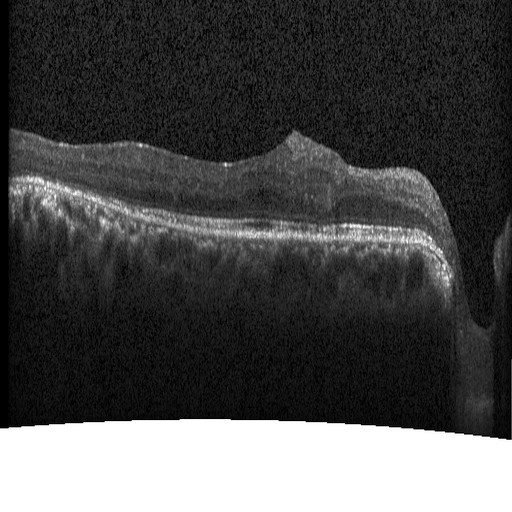 Macular OCT: DME.